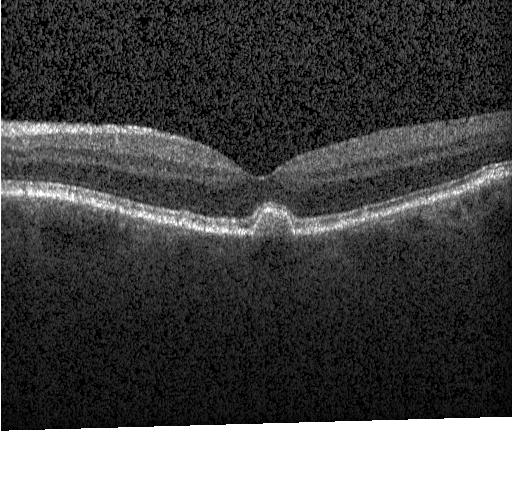

Impression: multiple drusen.